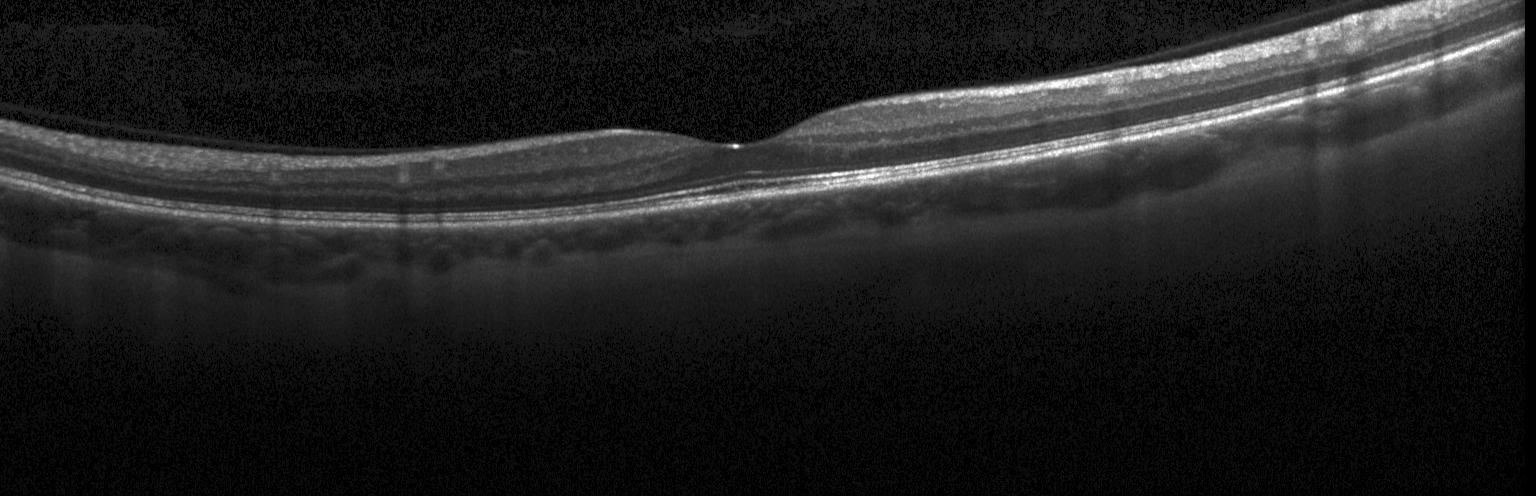 Spectral-domain OCT B-scan: neither CNV, DME, nor drusen.